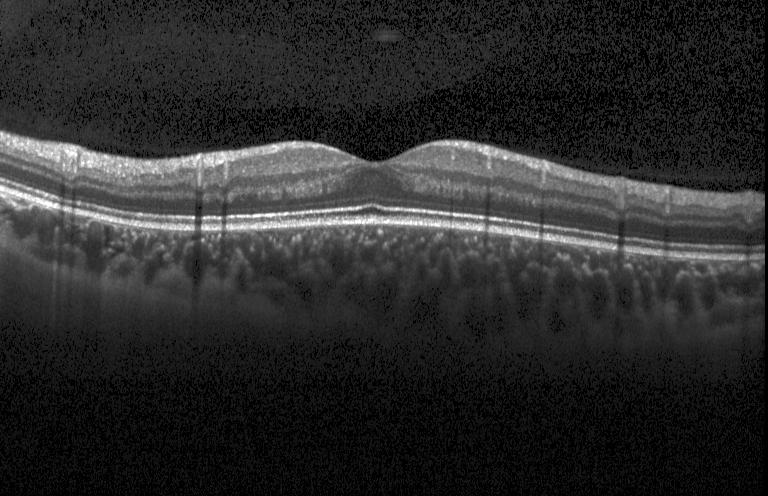

Impression: no choroidal neovascularization, diabetic macular edema, or drusen.